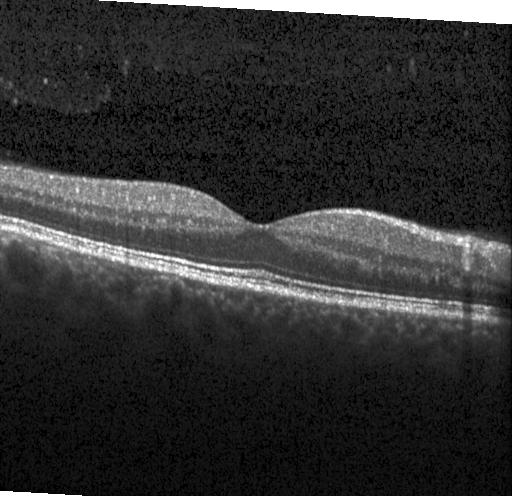

OCT line scan
Assessment: neither CNV, DME, nor drusen.